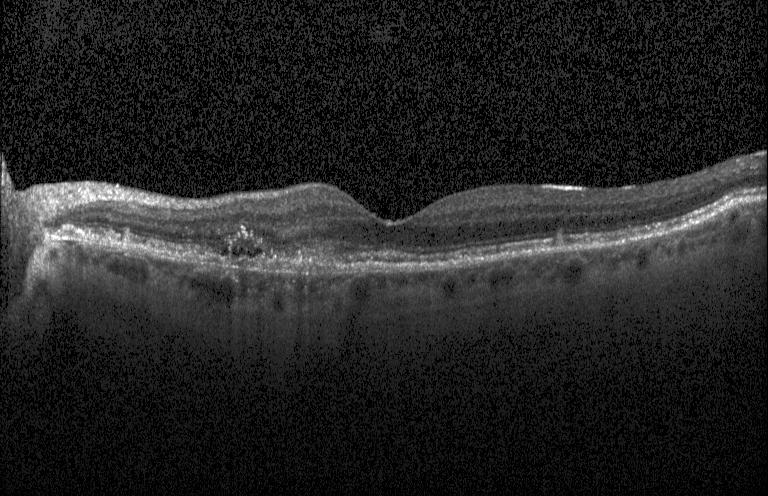

OCT line scan.
Impression: a choroidal neovascular membrane.